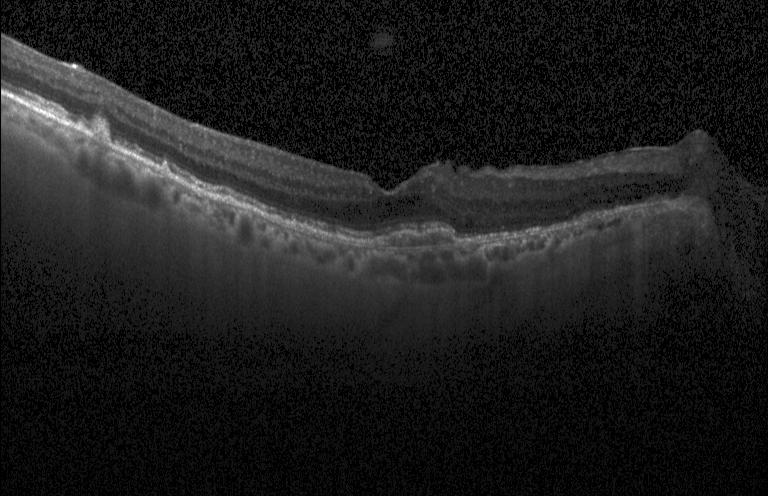
Through the macula, optical coherence tomography scan.
Diagnosis: a choroidal neovascular membrane.